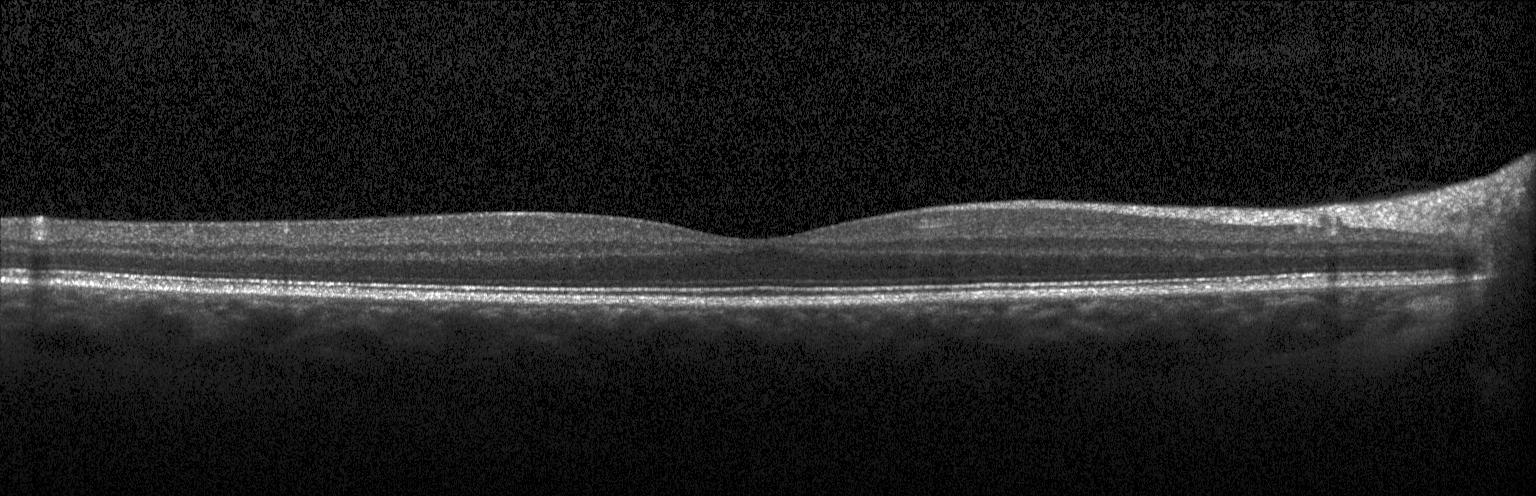
Optical coherence tomography scan; macular scan; Heidelberg Spectralis OCT system — Diagnosis: no evidence of choroidal neovascularization, diabetic macular edema, or drusen.